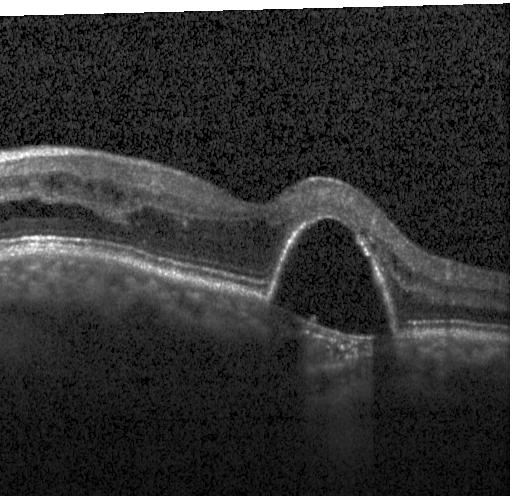
Through the macula; instrument: Heidelberg Spectralis; SD-OCT; retinal OCT B-scan.
OCT finding: choroidal neovascularization.